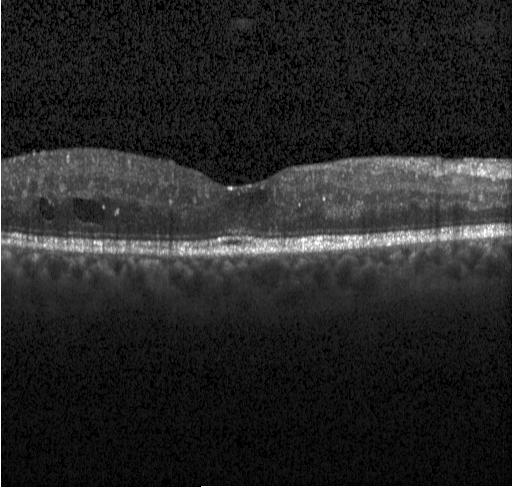
Spectral-domain OCT, retinal OCT cross-section.
Dx: diabetic macular edema.